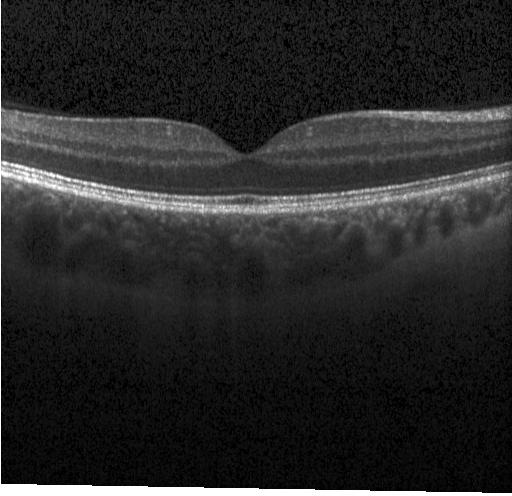

Spectral-domain OCT · optical coherence tomography scan · horizontal scan through the fovea. This B-scan demonstrates neither choroidal neovascularization, diabetic macular edema, nor drusen.